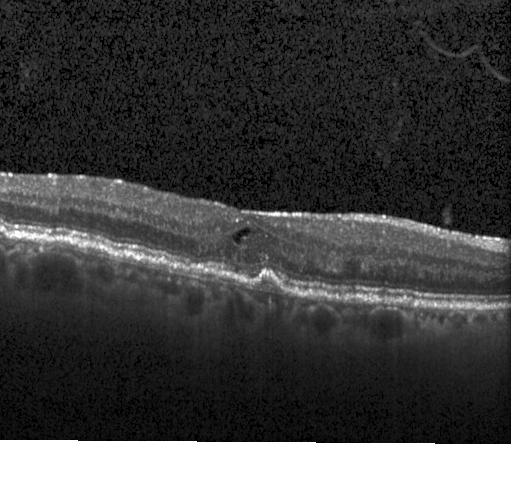
OCT B-scan · through the macula
Diagnosis: a choroidal neovascular membrane.